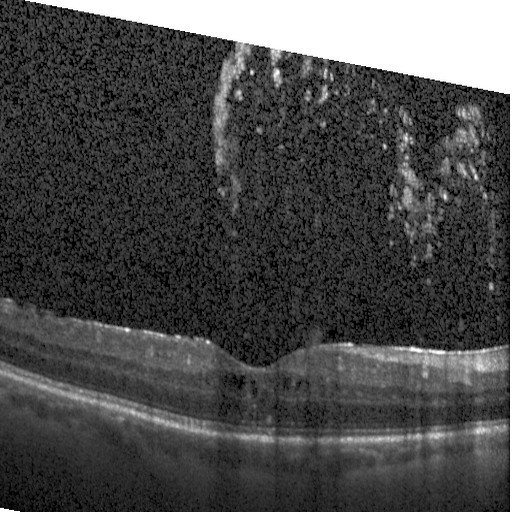
Retinal OCT cross-section; spectral-domain OCT; macular scan; Heidelberg Spectralis OCT system
Dx: DME.